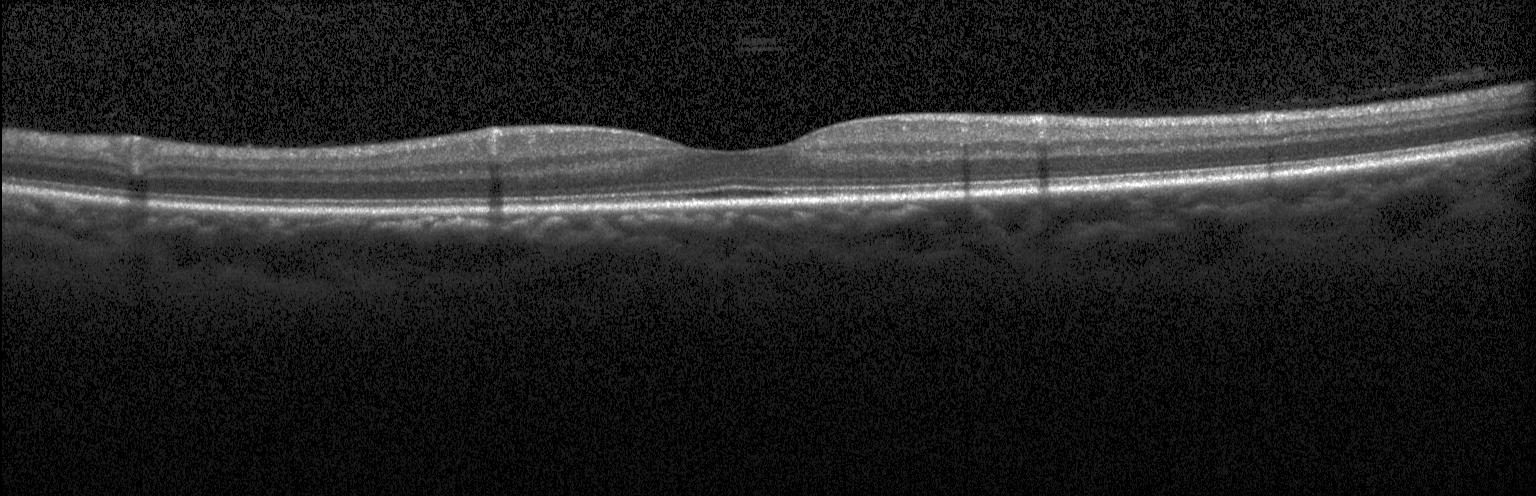
Instrument: Heidelberg Spectralis; optical coherence tomography B-scan
Dx: no choroidal neovascularization, diabetic macular edema, or drusen.